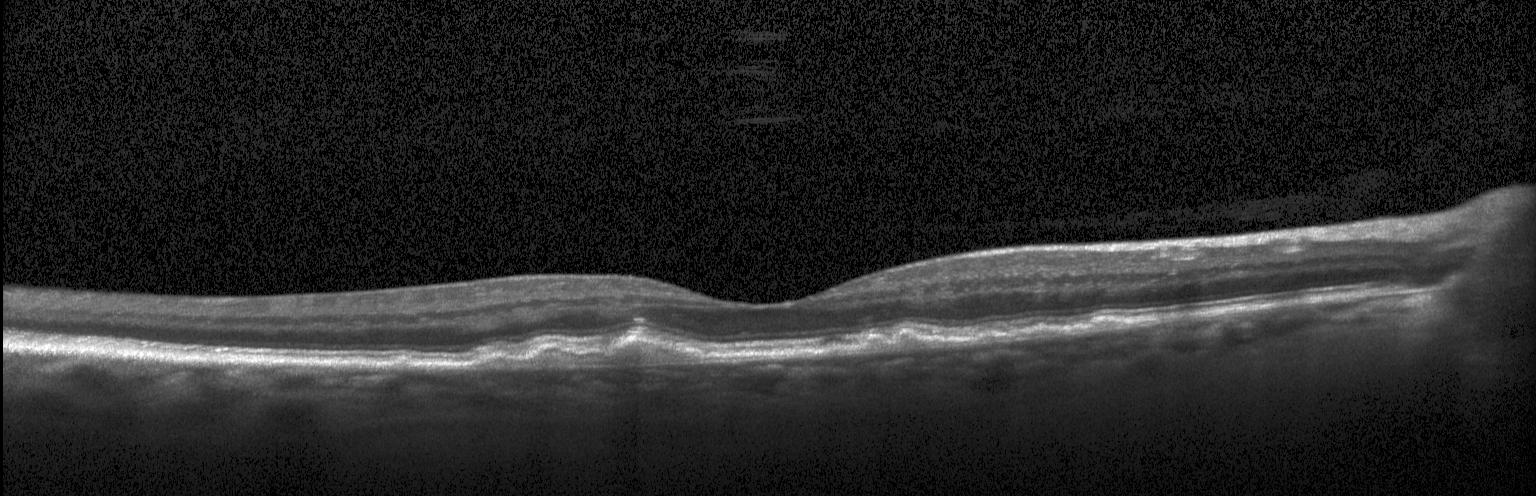 OCT finding: drusen.